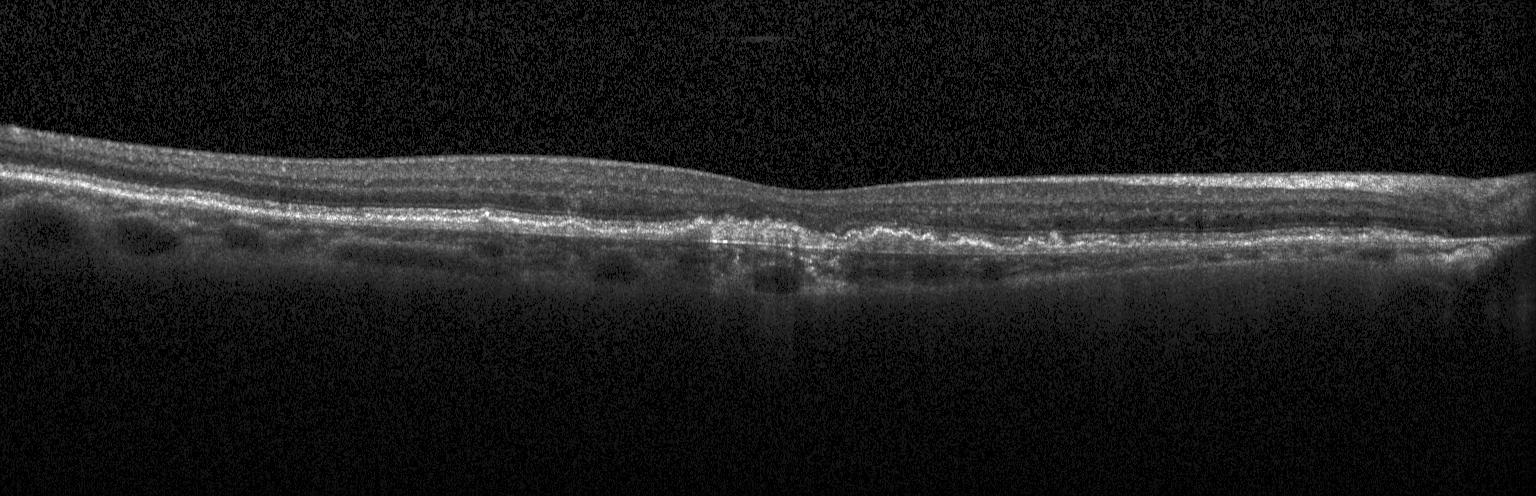
Optical coherence tomography scan
The scan shows choroidal neovascularization.